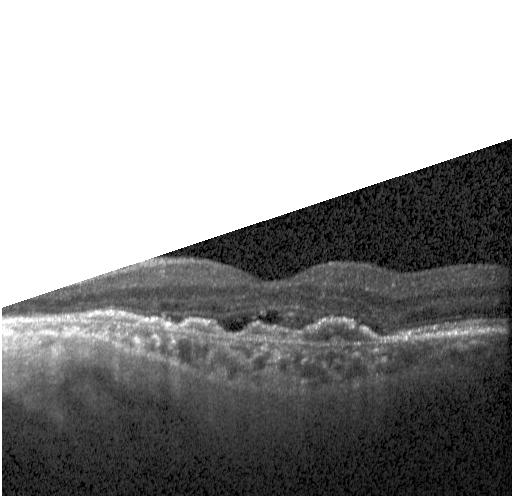 Macular OCT: choroidal neovascularization (CNV).